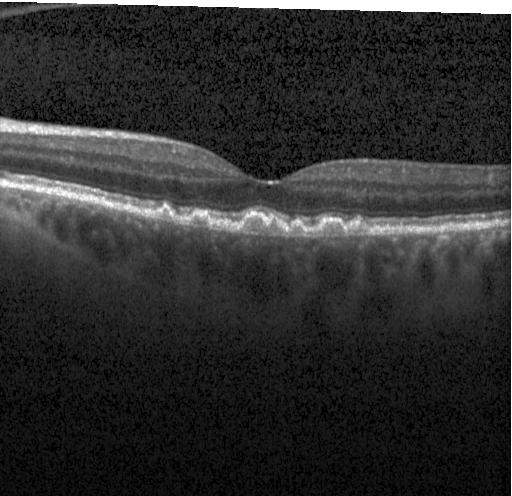
OCT line scan — Macular OCT: multiple drusen.